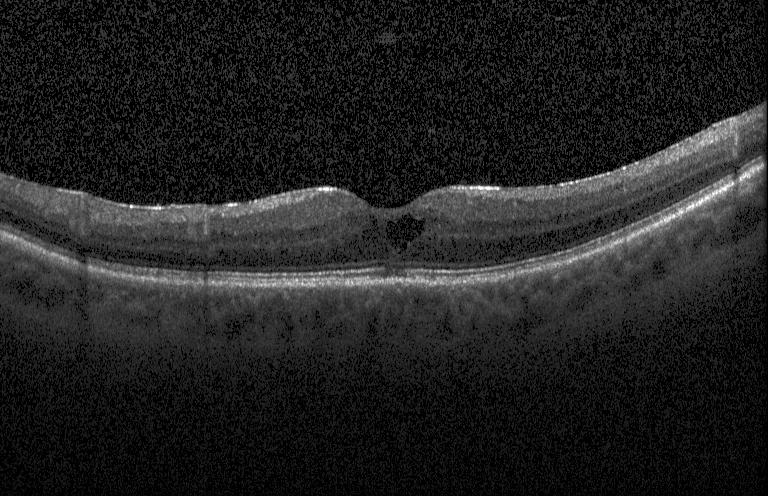

Retinal OCT cross-section
Macular OCT: diabetic macular edema.